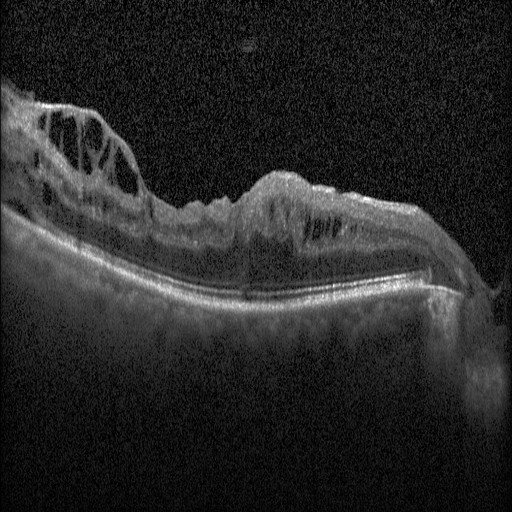
Macular scan; retinal OCT cross-section; SD-OCT; Heidelberg Spectralis.
Finding: diabetic macular edema (DME).